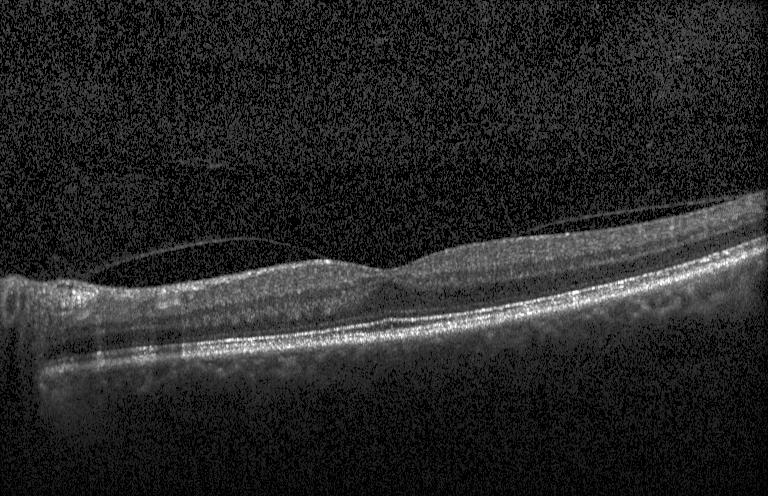
No choroidal neovascularization, diabetic macular edema, or drusen.